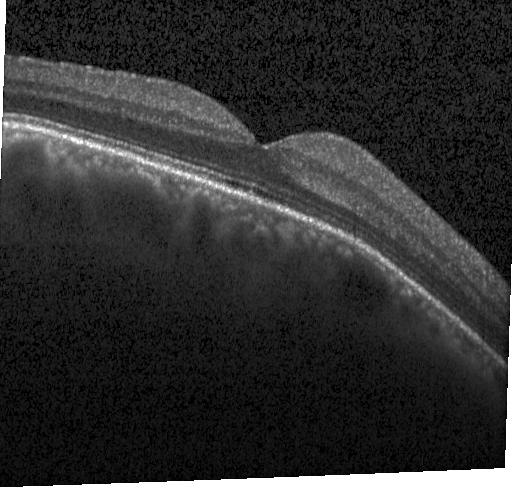
Spectral-domain OCT B-scan: no choroidal neovascularization, diabetic macular edema, or drusen.